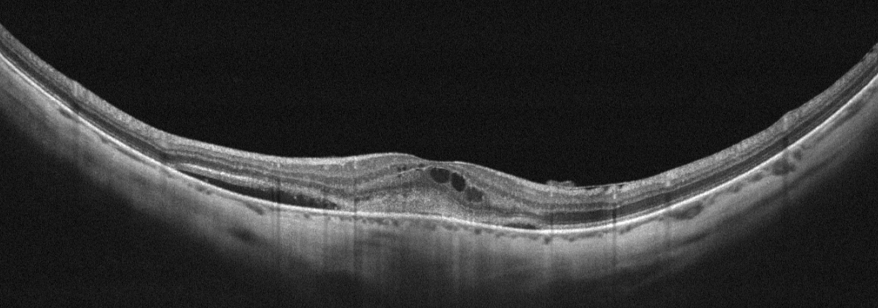

OCT line scan — Assessment: age-related macular degeneration.